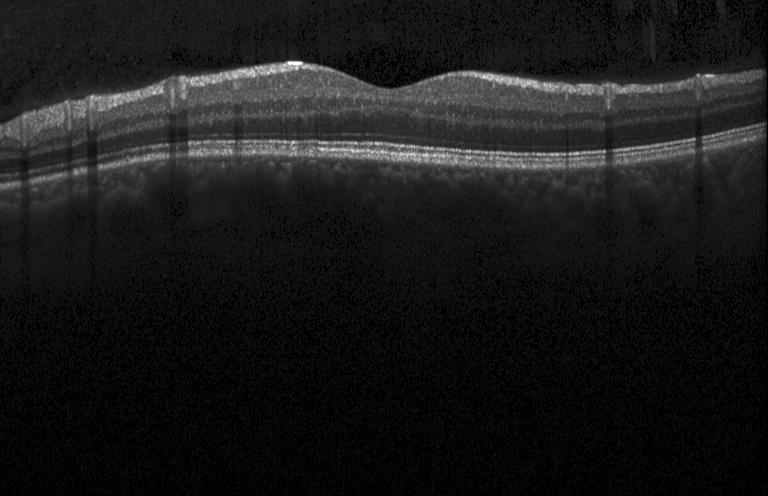

Instrument: Heidelberg Spectralis · OCT line scan.
Finding: no evidence of choroidal neovascularization, diabetic macular edema, or drusen.